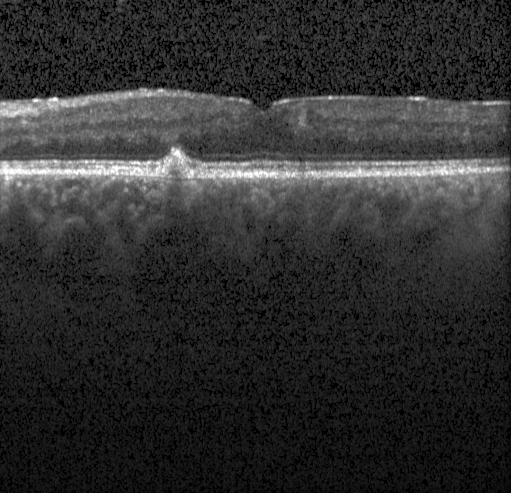
Centered on the fovea. Retinal OCT B-scan — Finding: sub-RPE drusenoid deposits.